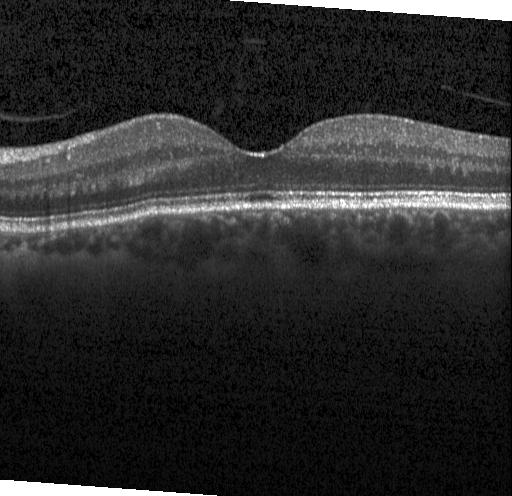

Fovea-centered · OCT line scan · SD-OCT.
This B-scan demonstrates no choroidal neovascularization, no diabetic macular edema, and no drusen.